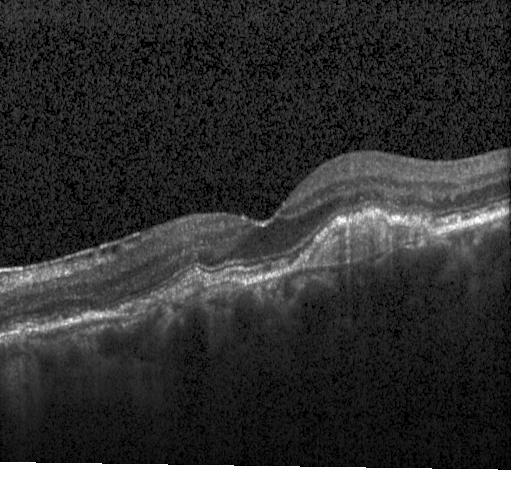

OCT B-scan, instrument: Heidelberg Spectralis. Finding: choroidal neovascularization (CNV).